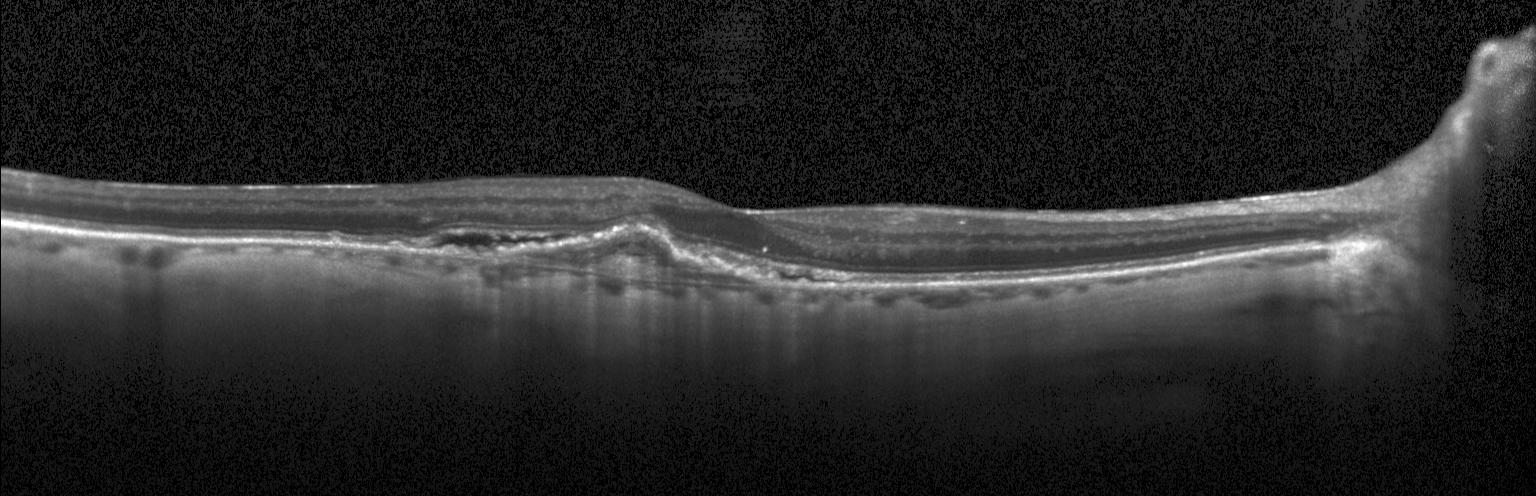

Heidelberg Spectralis · retinal OCT B-scan
Finding: a choroidal neovascular membrane.